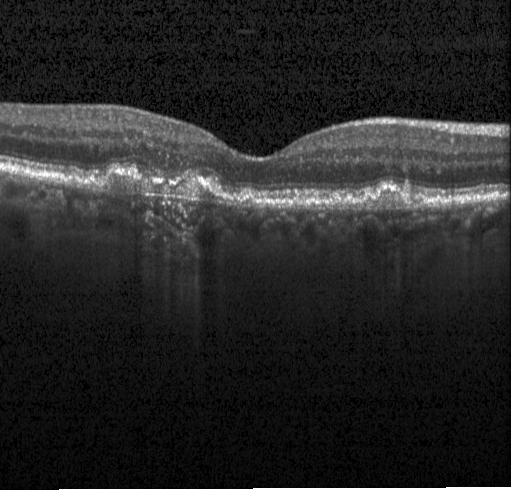

Optical coherence tomography B-scan.
Impression: a choroidal neovascular membrane.